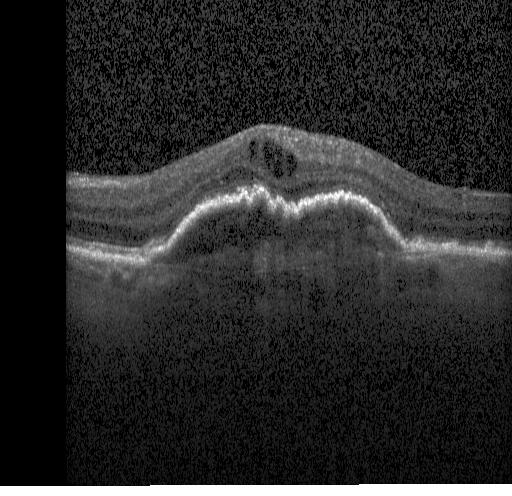
OCT B-scan · Heidelberg Spectralis OCT system
Macular OCT: CNV.